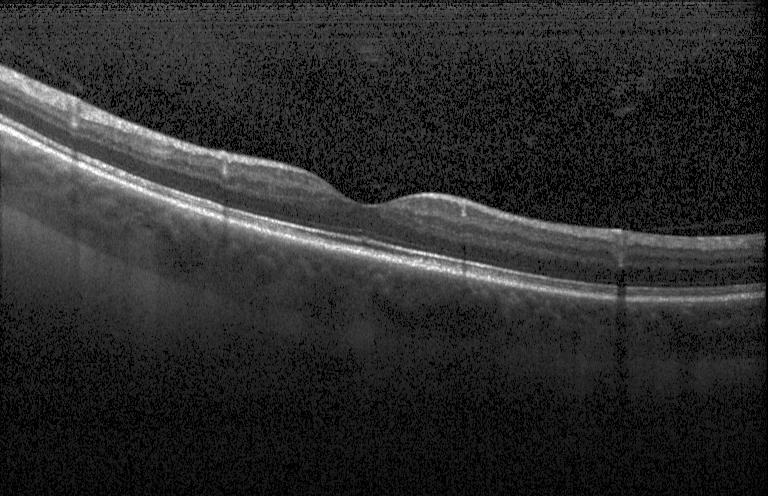
Optical coherence tomography scan.
Assessment: no evidence of choroidal neovascularization, diabetic macular edema, or drusen.